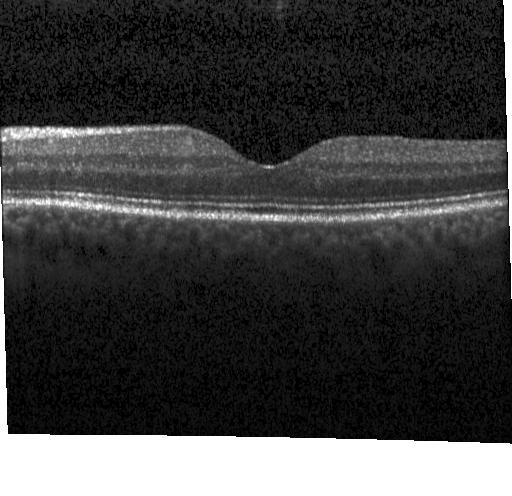 Horizontal scan through the fovea; OCT line scan; spectral-domain OCT. Diagnosis: neither choroidal neovascularization, diabetic macular edema, nor drusen.